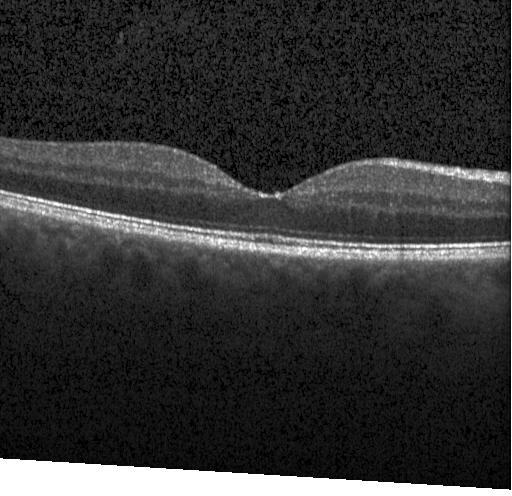

Optical coherence tomography scan · acquired on a Heidelberg Spectralis.
Finding: neither choroidal neovascularization, diabetic macular edema, nor drusen.